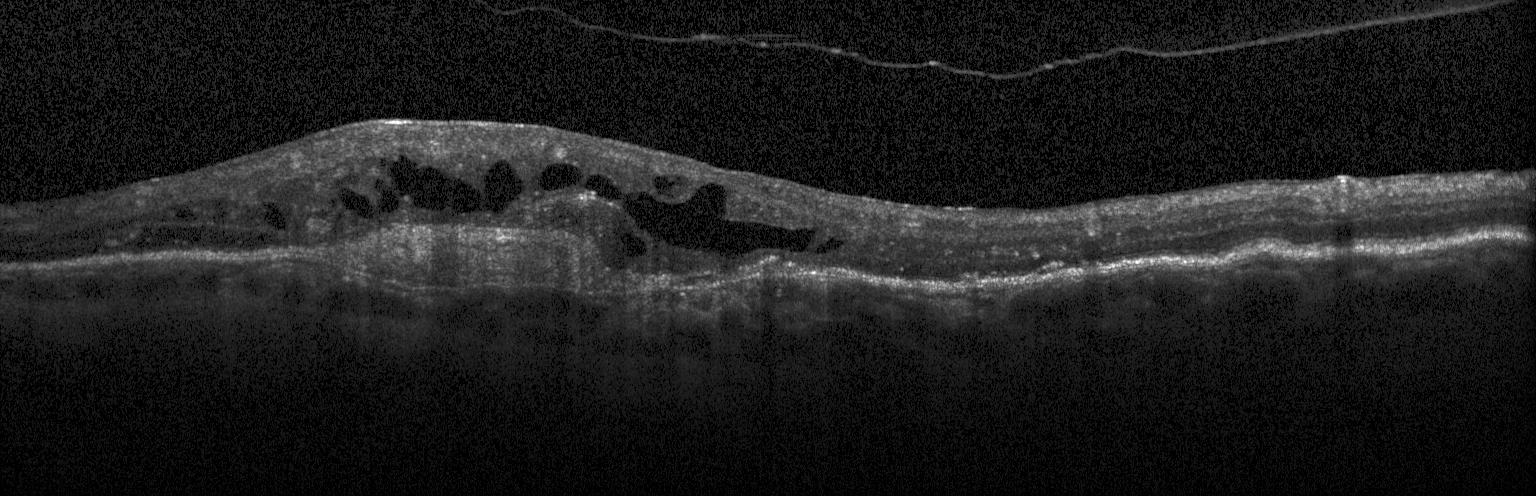

Acquired on a Heidelberg Spectralis. Horizontal scan through the fovea. Spectral-domain OCT. OCT line scan.
Dx: choroidal neovascularization (CNV).